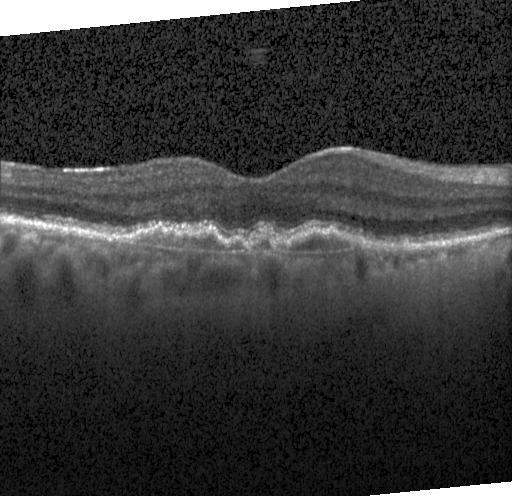 OCT B-scan
Choroidal neovascularization.